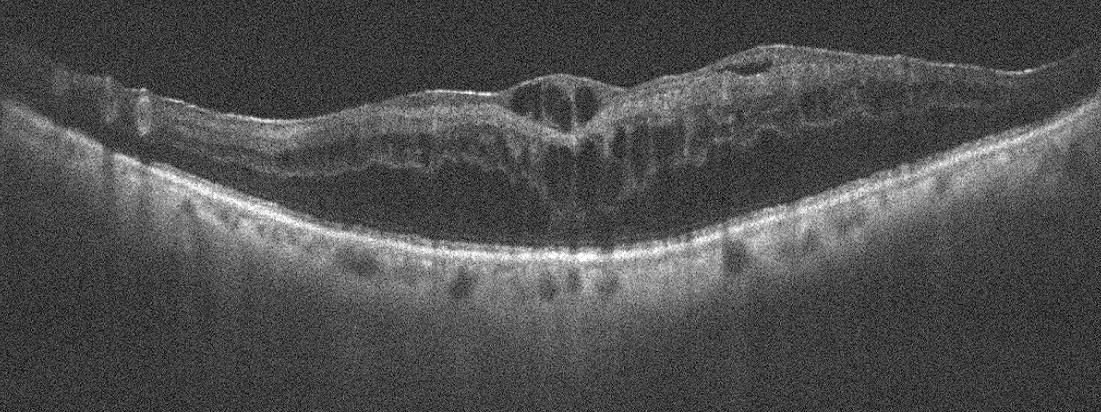
Acquired on an Optovue Avanti RTVue XR, OCT B-scan — Finding: retinal vein occlusion (RVO).